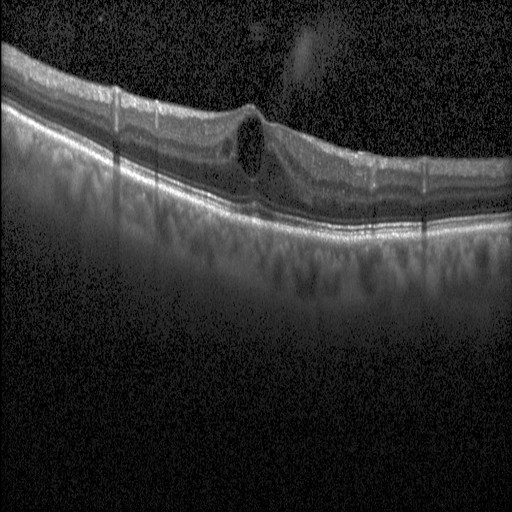 Impression: diabetic macular edema (DME).